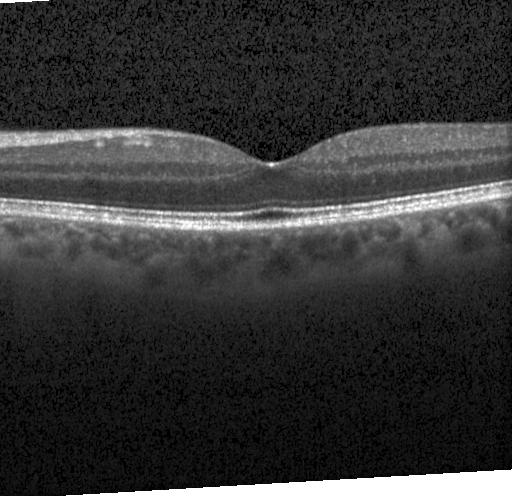 Retinal OCT cross-section
The scan shows no evidence of choroidal neovascularization, diabetic macular edema, or drusen.